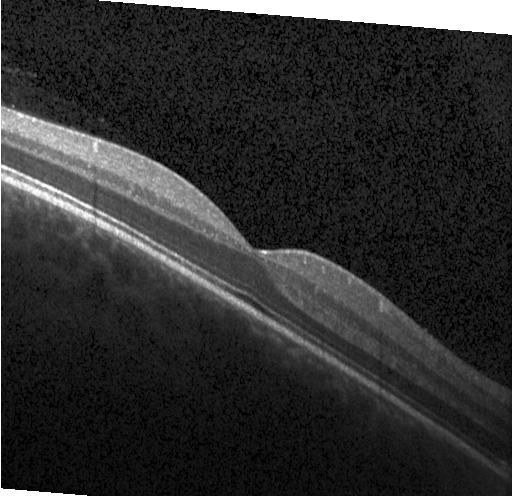 Optical coherence tomography scan — This B-scan demonstrates no evidence of choroidal neovascularization, diabetic macular edema, or drusen.